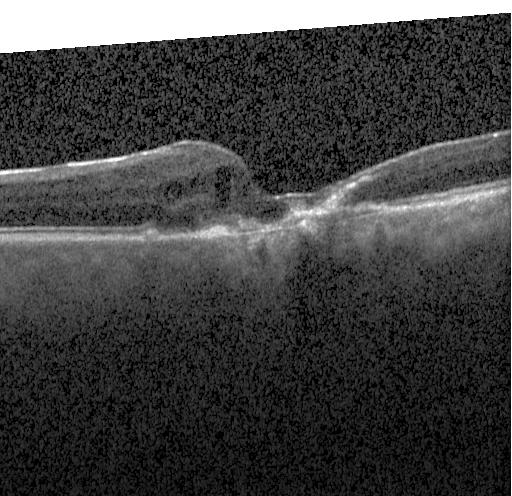
Diagnosis: a choroidal neovascular membrane.